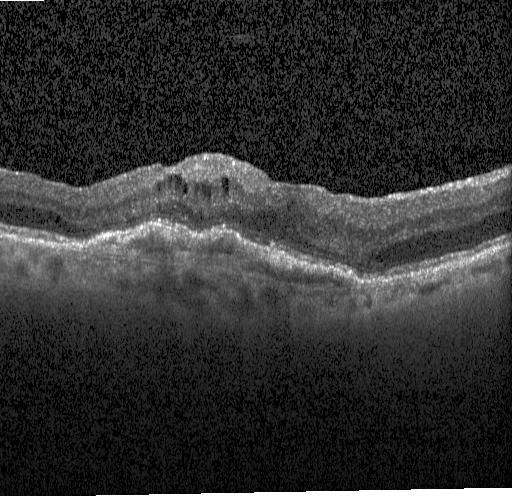
Optical coherence tomography B-scan; horizontal scan through the fovea — Diagnosis: a choroidal neovascular membrane.